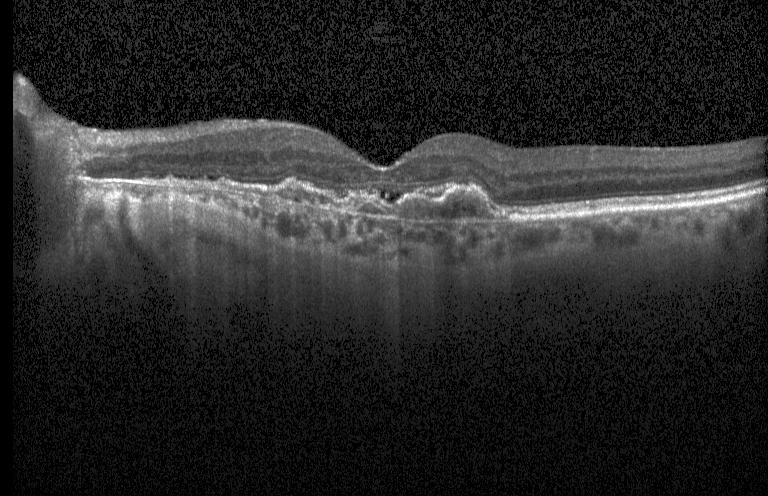 Optical coherence tomography scan. SD-OCT. Fovea-centered. Heidelberg Spectralis OCT system
The scan shows a choroidal neovascular membrane.